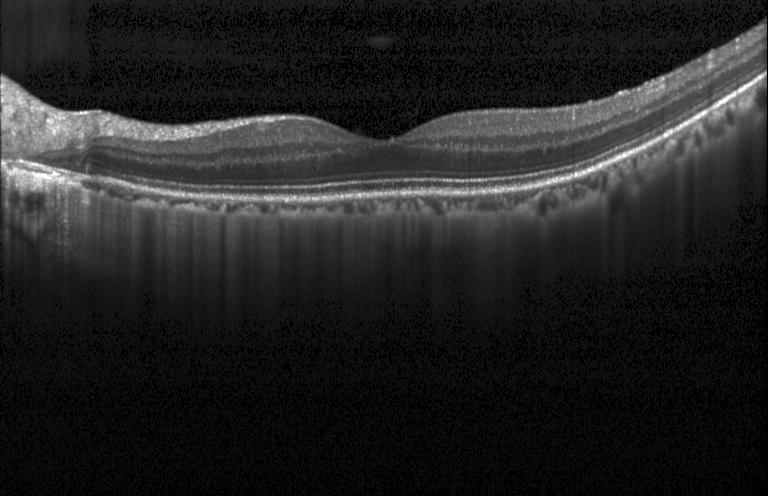 OCT B-scan showing neither choroidal neovascularization, diabetic macular edema, nor drusen.